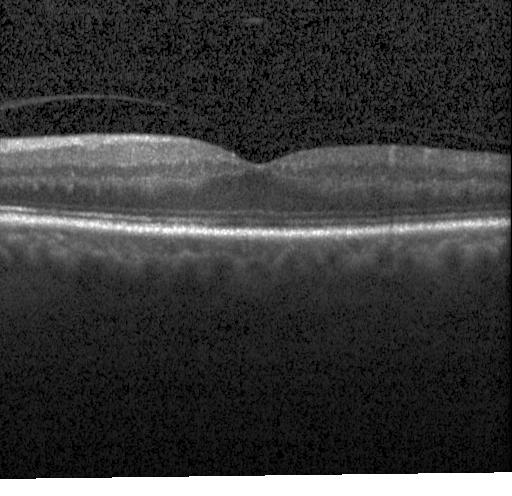 Impression: no CNV, no DME, and no drusen.